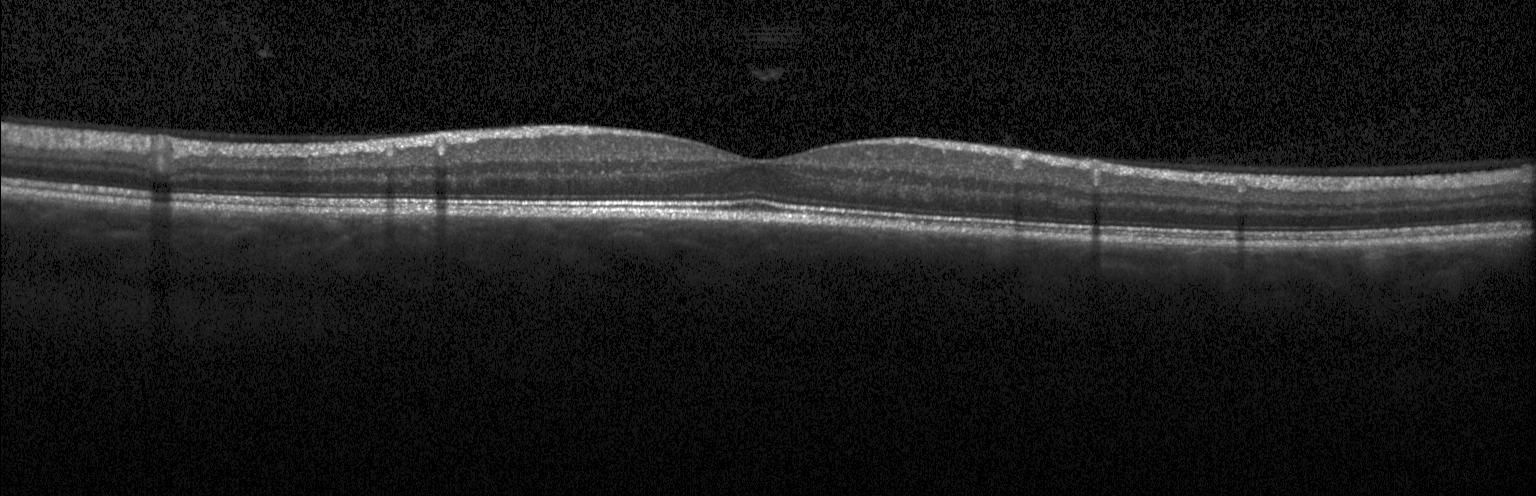
Impression: neither choroidal neovascularization, diabetic macular edema, nor drusen.